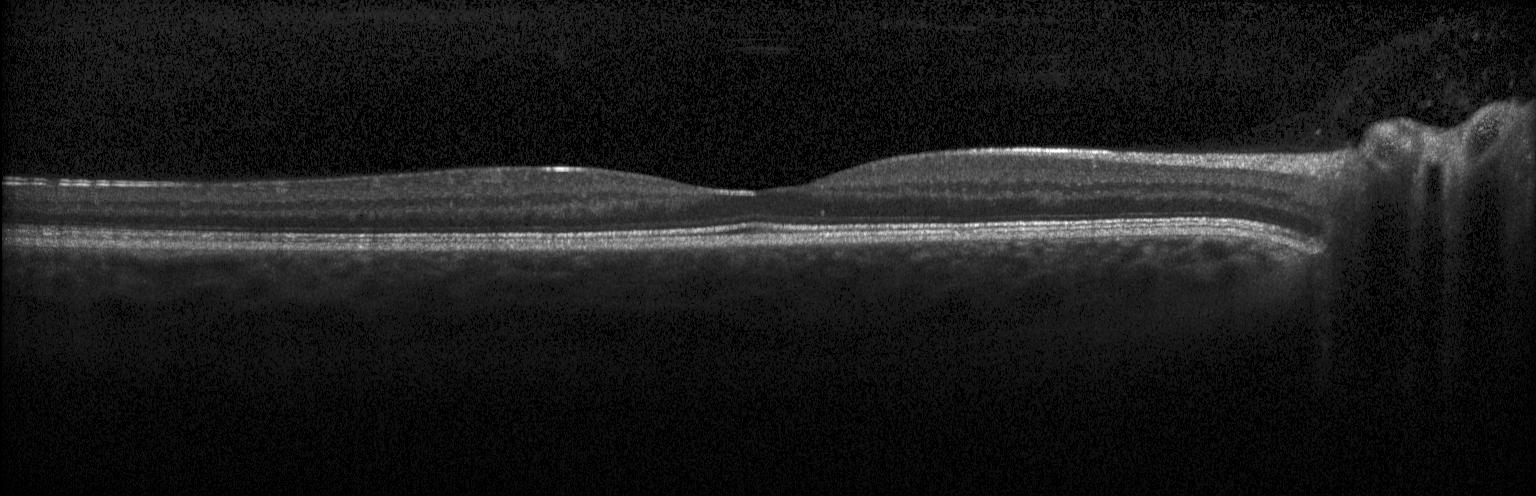

SD-OCT; retinal OCT B-scan; Heidelberg Spectralis; centered on the fovea — Assessment: no evidence of choroidal neovascularization, diabetic macular edema, or drusen.